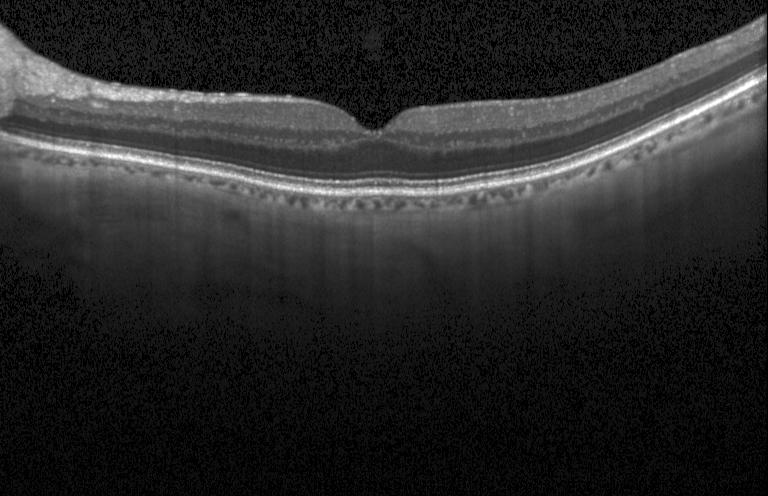

Macular OCT: no CNV, DME, or drusen.